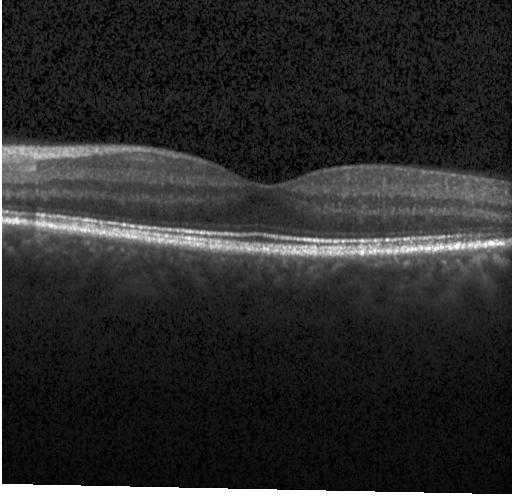
Diagnosis: no choroidal neovascularization, no diabetic macular edema, and no drusen.